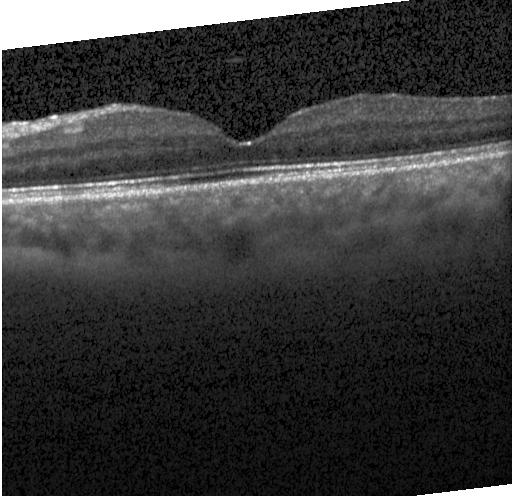

Spectral-domain optical coherence tomography. Optical coherence tomography B-scan.
Macular OCT: no choroidal neovascularization, no diabetic macular edema, and no drusen.